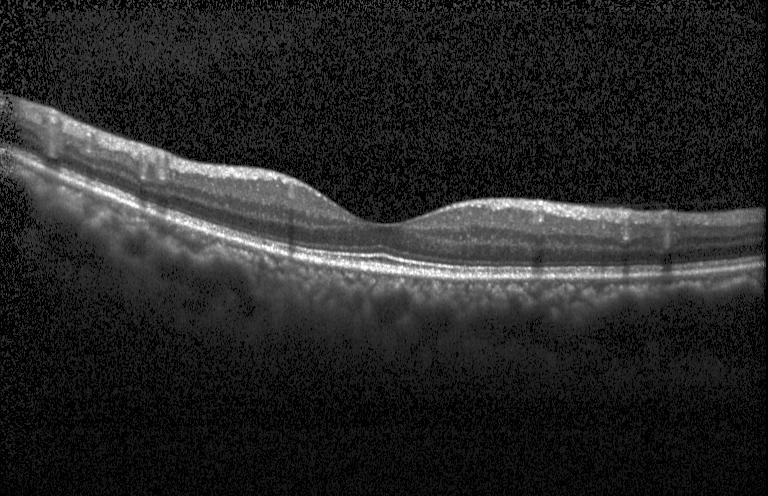 Assessment: no evidence of choroidal neovascularization, diabetic macular edema, or drusen.